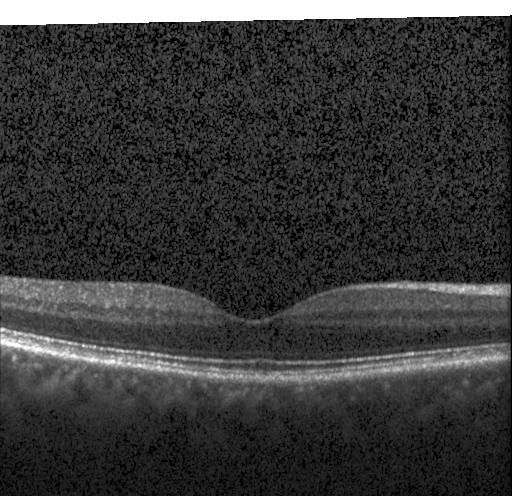 Fovea-centered, OCT line scan — This B-scan demonstrates neither choroidal neovascularization, diabetic macular edema, nor drusen.